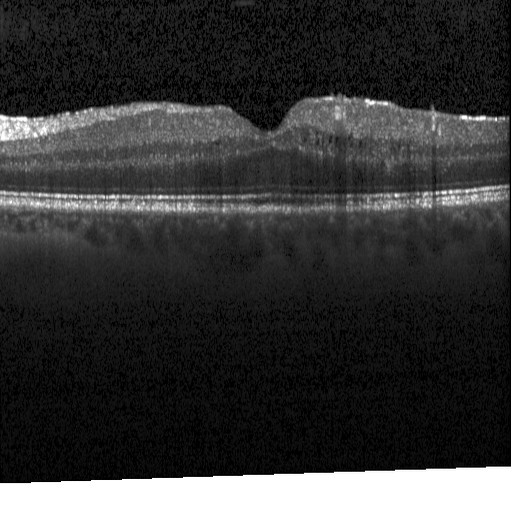

OCT scan showing diabetic macular edema.